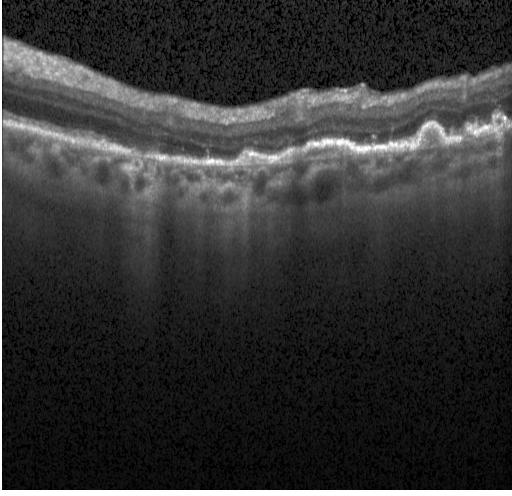
Retinal OCT cross-section; SD-OCT. Finding: a choroidal neovascular membrane.